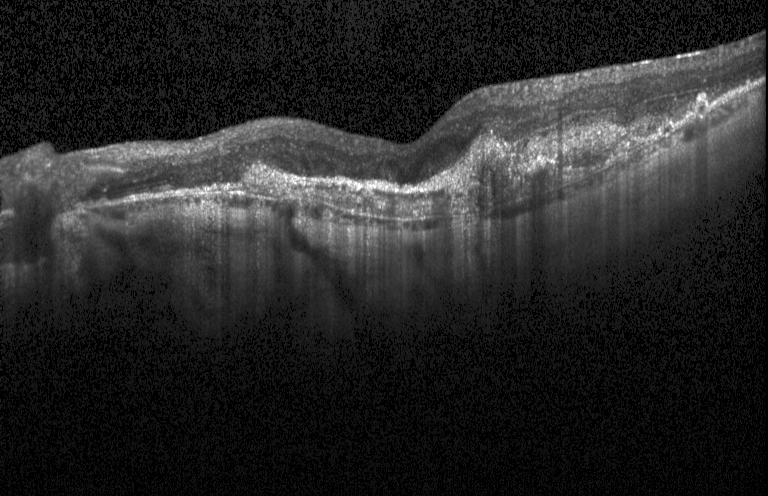
A choroidal neovascular membrane.